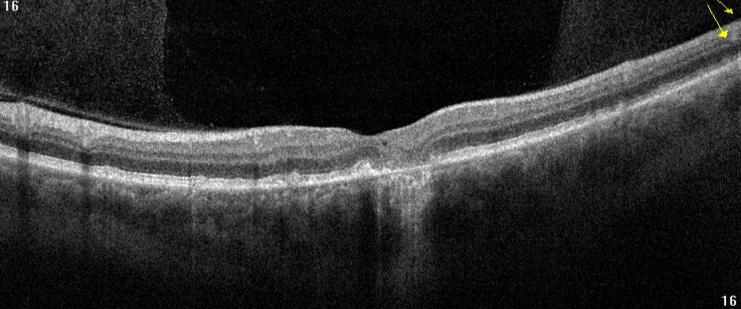 OCT line scan · through the macula · acquired on an Optovue Avanti RTVue XR
This B-scan demonstrates AMD.